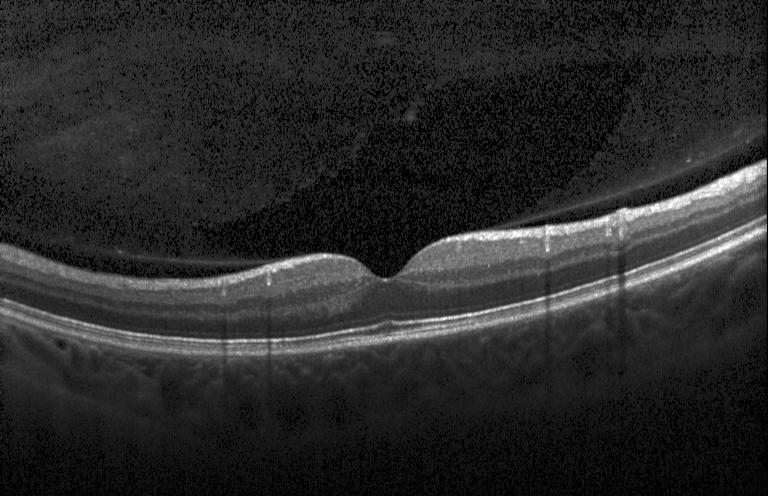 Macular OCT: no CNV, no DME, and no drusen.